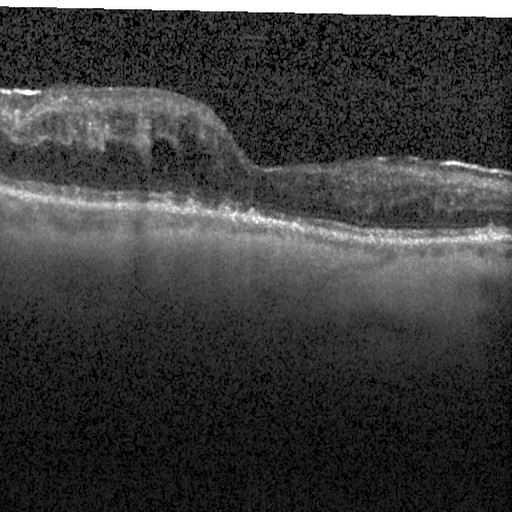
Horizontal scan through the fovea · spectral-domain OCT · OCT B-scan. Finding: diabetic macular edema (DME).